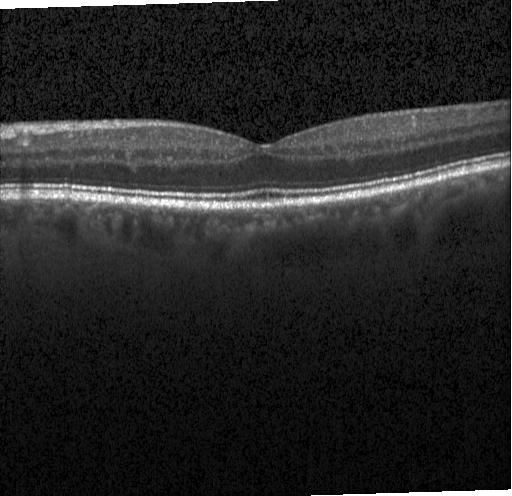 Impression: no evidence of CNV, DME, or drusen.